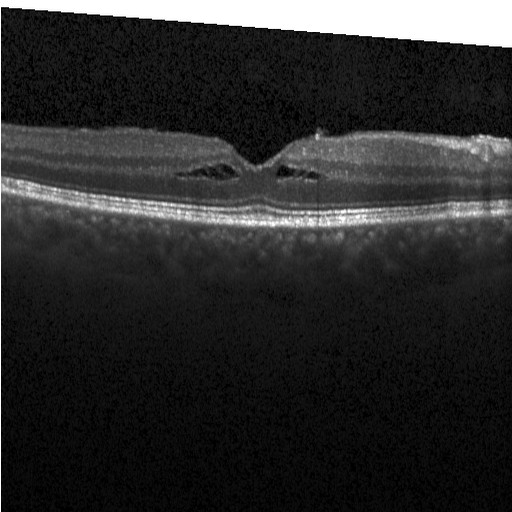

Macular scan; optical coherence tomography scan. Macular OCT: DME.